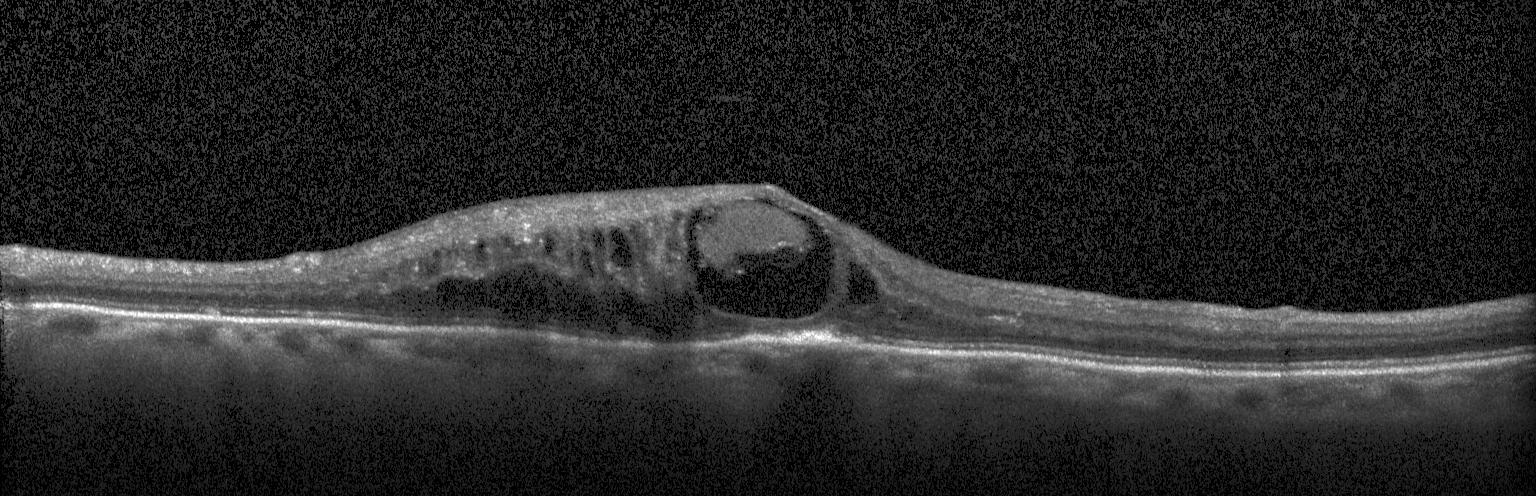 Dx: diabetic macular edema (DME).